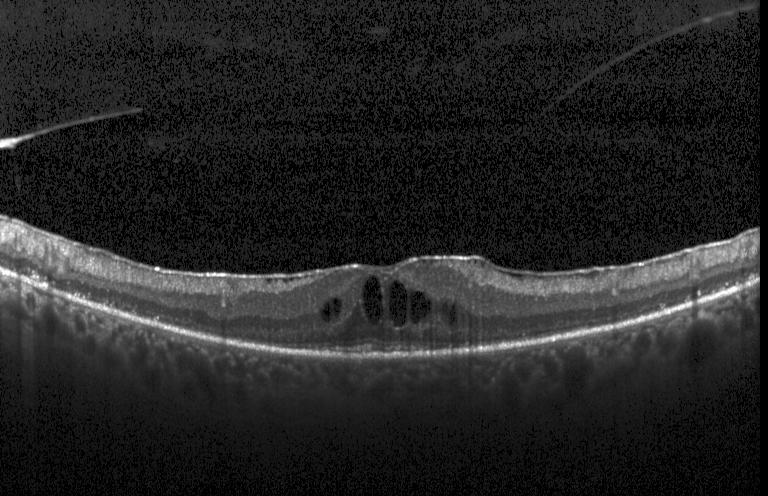

Heidelberg Spectralis OCT system, optical coherence tomography B-scan. Dx: diabetic macular edema.